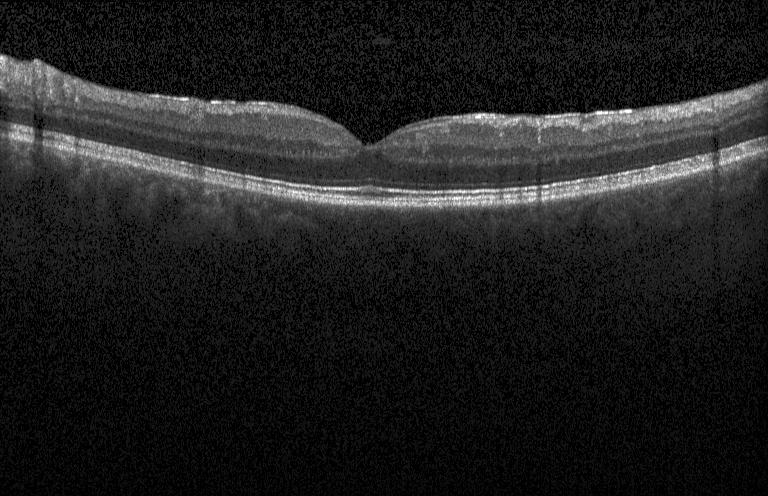 No choroidal neovascularization, no diabetic macular edema, and no drusen.